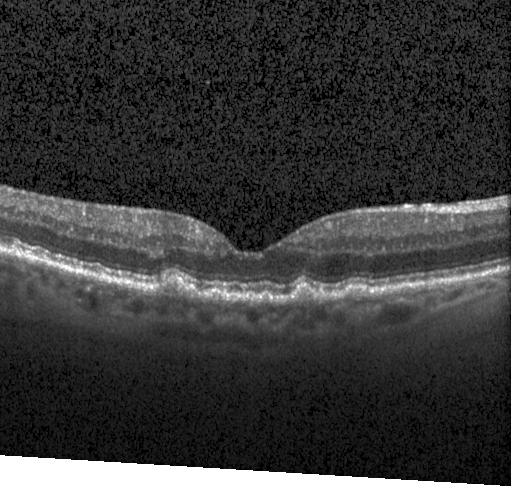
Acquired on a Heidelberg Spectralis · OCT line scan.
Finding: multiple drusen.